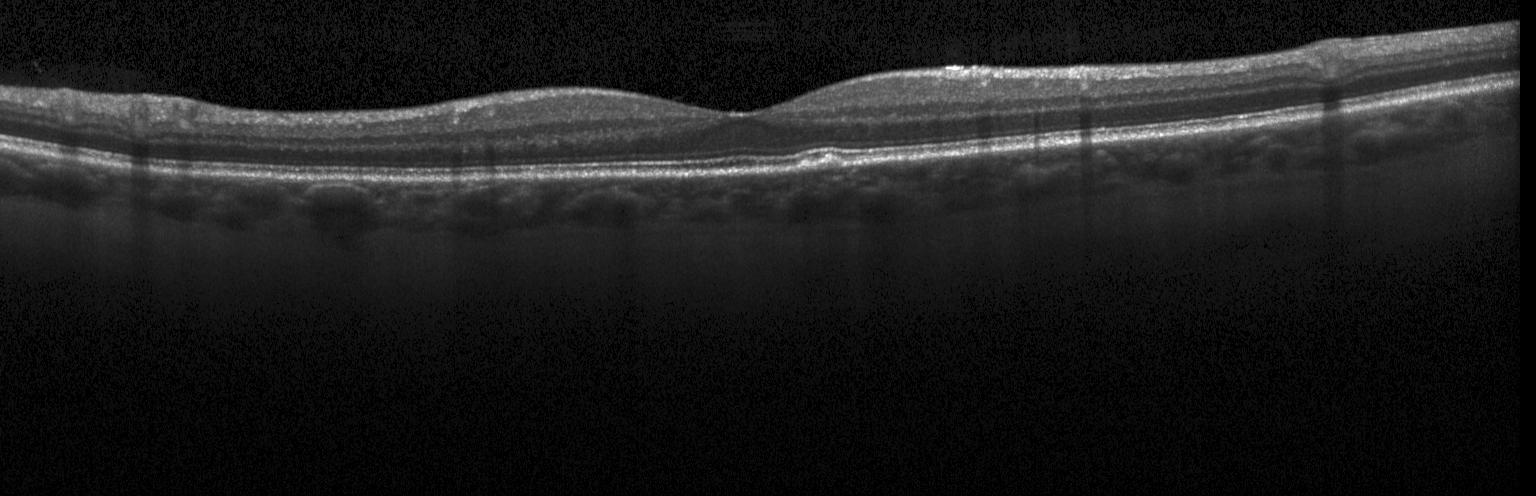 Finding: multiple drusen.